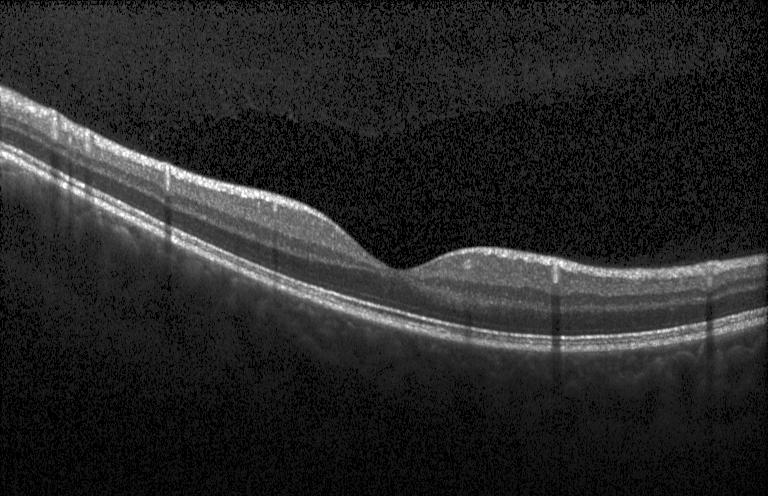

Diagnosis: no CNV, DME, or drusen.